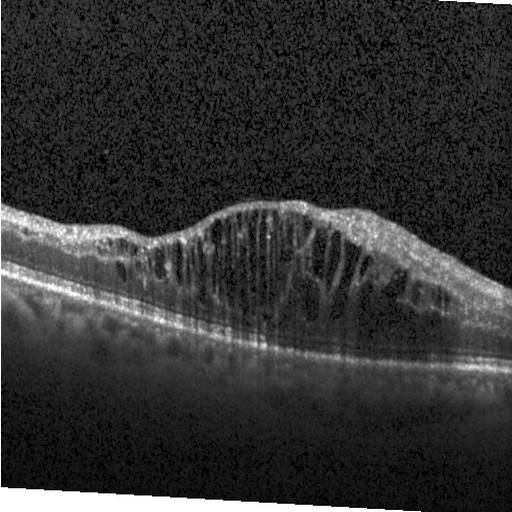
Instrument: Heidelberg Spectralis. OCT line scan. Fovea-centered
OCT finding: DME.